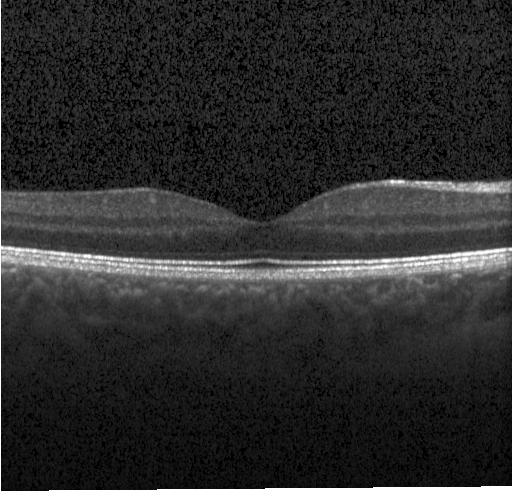

Neither choroidal neovascularization, diabetic macular edema, nor drusen.